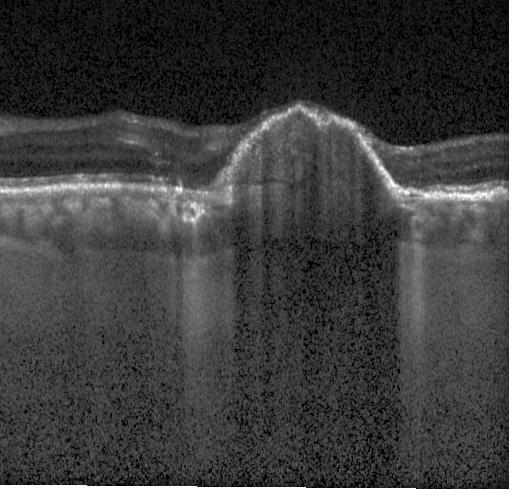
Finding: a choroidal neovascular membrane.